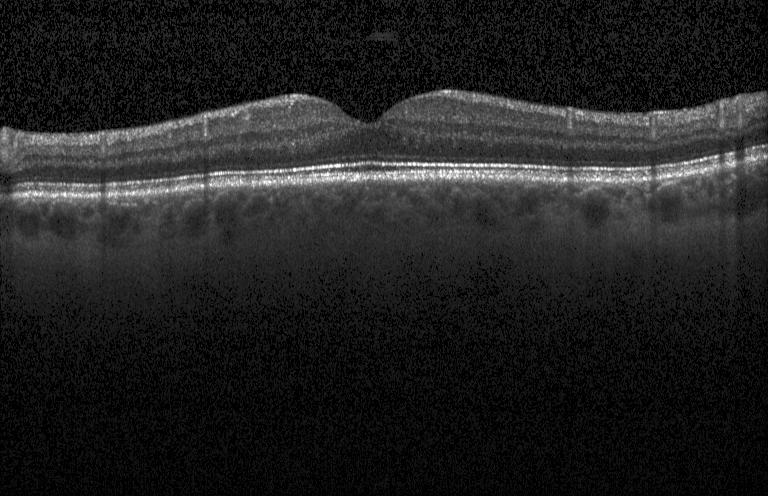 OCT finding: no choroidal neovascularization, diabetic macular edema, or drusen.